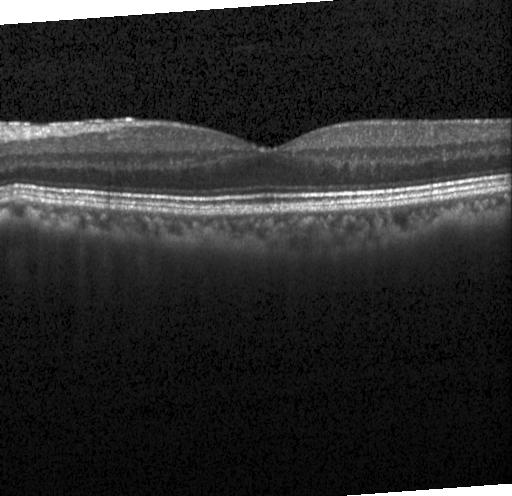

OCT B-scan — This B-scan demonstrates neither CNV, DME, nor drusen.